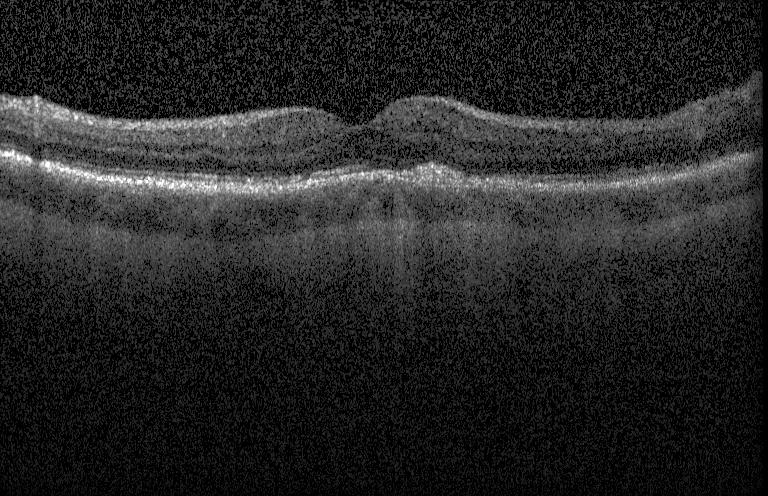
Assessment: a choroidal neovascular membrane.